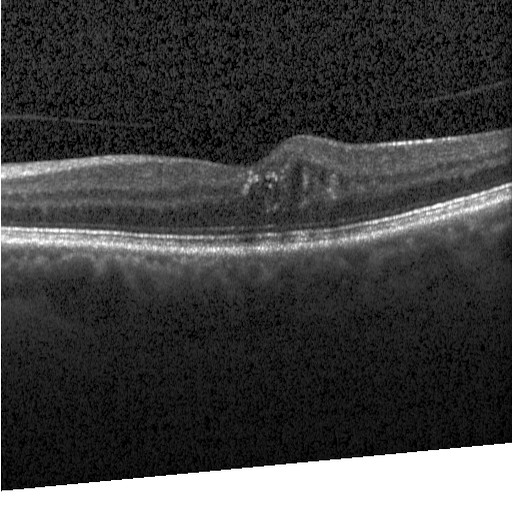 Macular OCT demonstrating DME.